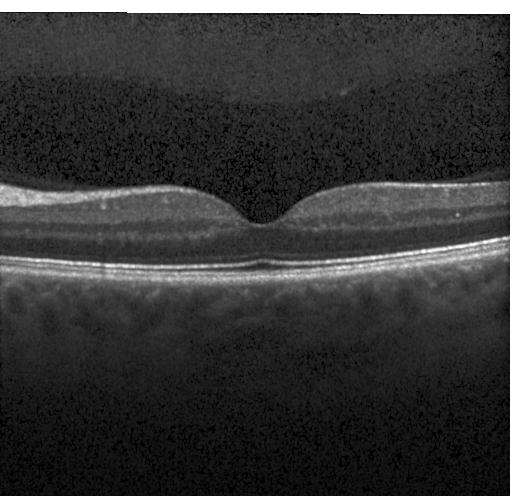

Through the macula. Instrument: Heidelberg Spectralis. Optical coherence tomography B-scan. Spectral-domain optical coherence tomography.
Diagnosis: no choroidal neovascularization, no diabetic macular edema, and no drusen.